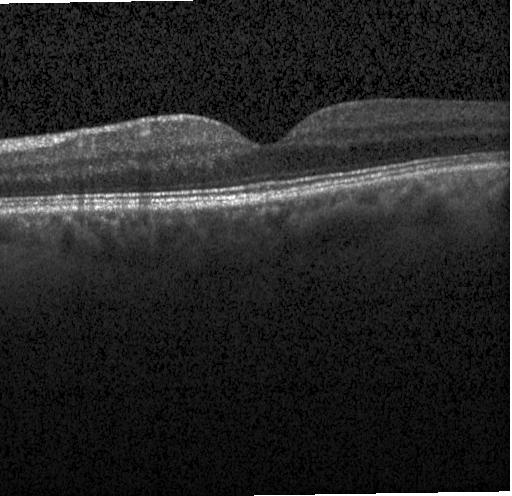
OCT finding: no choroidal neovascularization, diabetic macular edema, or drusen.